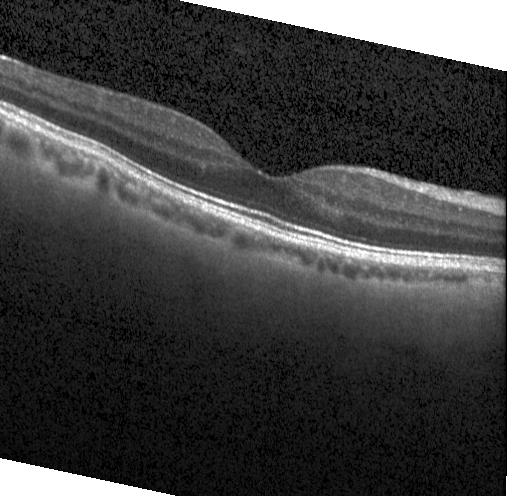 OCT line scan.
Finding: no evidence of choroidal neovascularization, diabetic macular edema, or drusen.